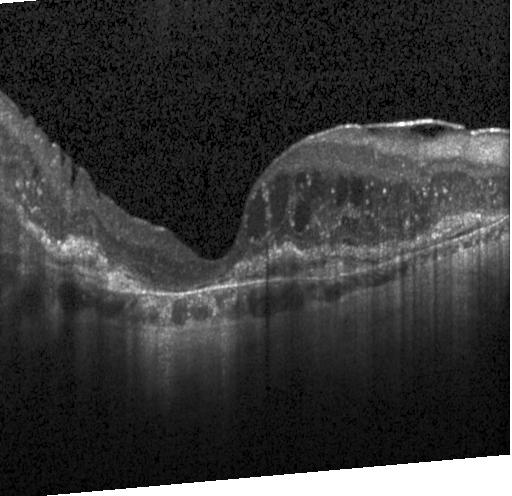
Optical coherence tomography scan.
This B-scan demonstrates a choroidal neovascular membrane.